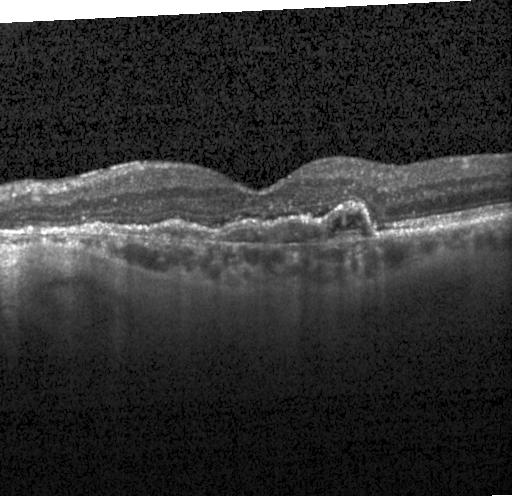
Diagnosis: choroidal neovascularization (CNV).